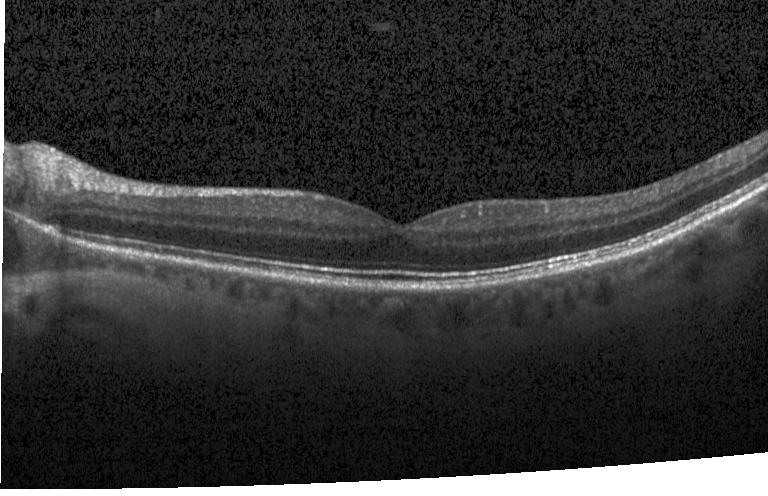

OCT finding: no choroidal neovascularization, diabetic macular edema, or drusen.